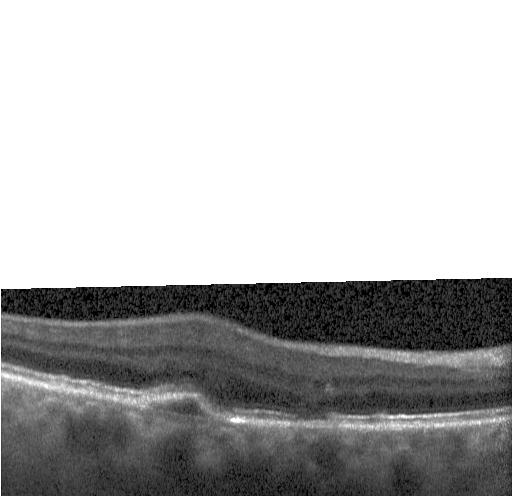

Horizontal scan through the fovea, spectral-domain optical coherence tomography, retinal OCT B-scan.
A choroidal neovascular membrane.